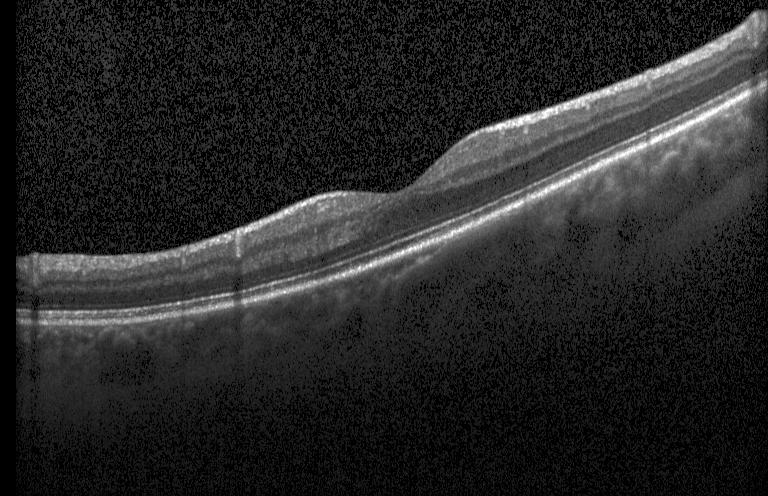

Retinal OCT cross-section showing neither choroidal neovascularization, diabetic macular edema, nor drusen.